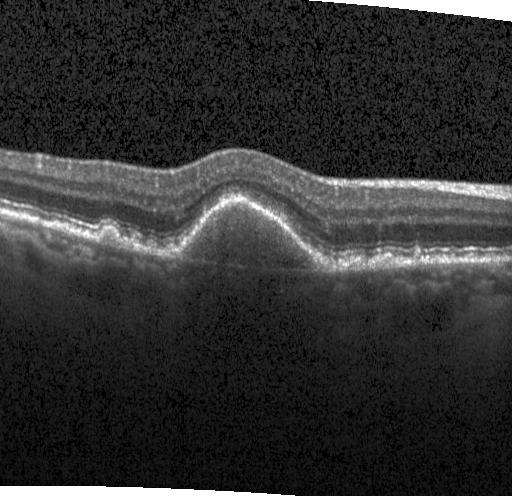

Acquired on a Heidelberg Spectralis; spectral-domain OCT; OCT B-scan; through the macula — CNV.